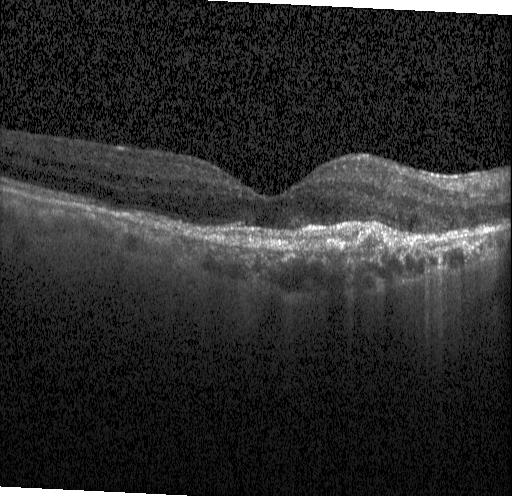

OCT line scan, spectral-domain optical coherence tomography — The scan shows a choroidal neovascular membrane.